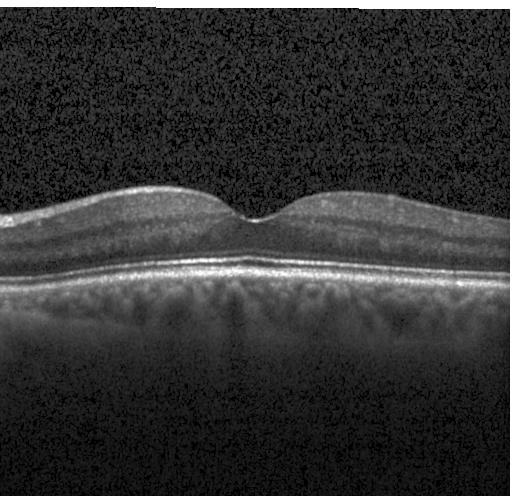
OCT line scan
Diagnosis: no choroidal neovascularization, no diabetic macular edema, and no drusen.